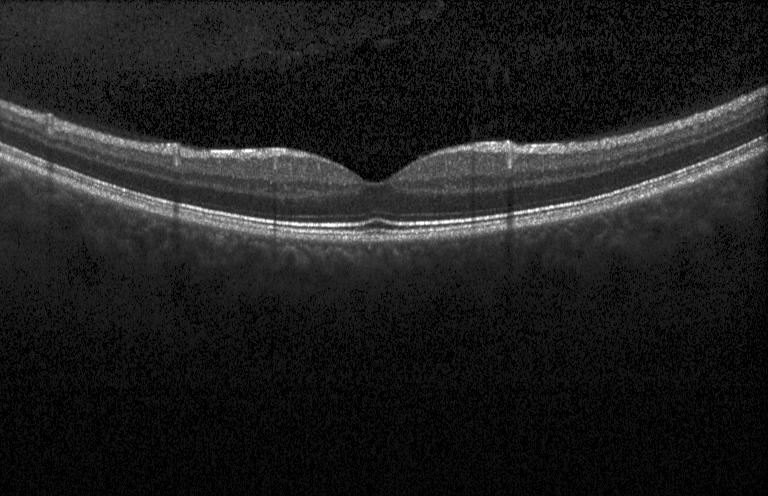

OCT B-scan
Assessment: no CNV, DME, or drusen.